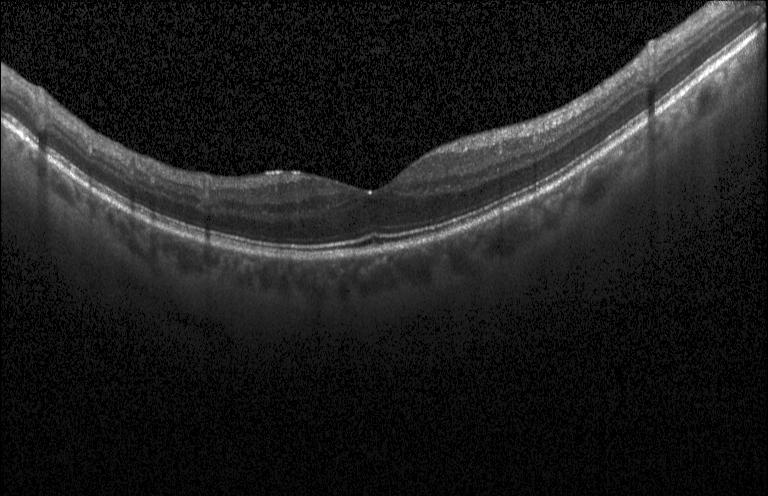

Spectral-domain optical coherence tomography · macular scan · Heidelberg Spectralis OCT system · retinal OCT B-scan.
OCT finding: no choroidal neovascularization, no diabetic macular edema, and no drusen.